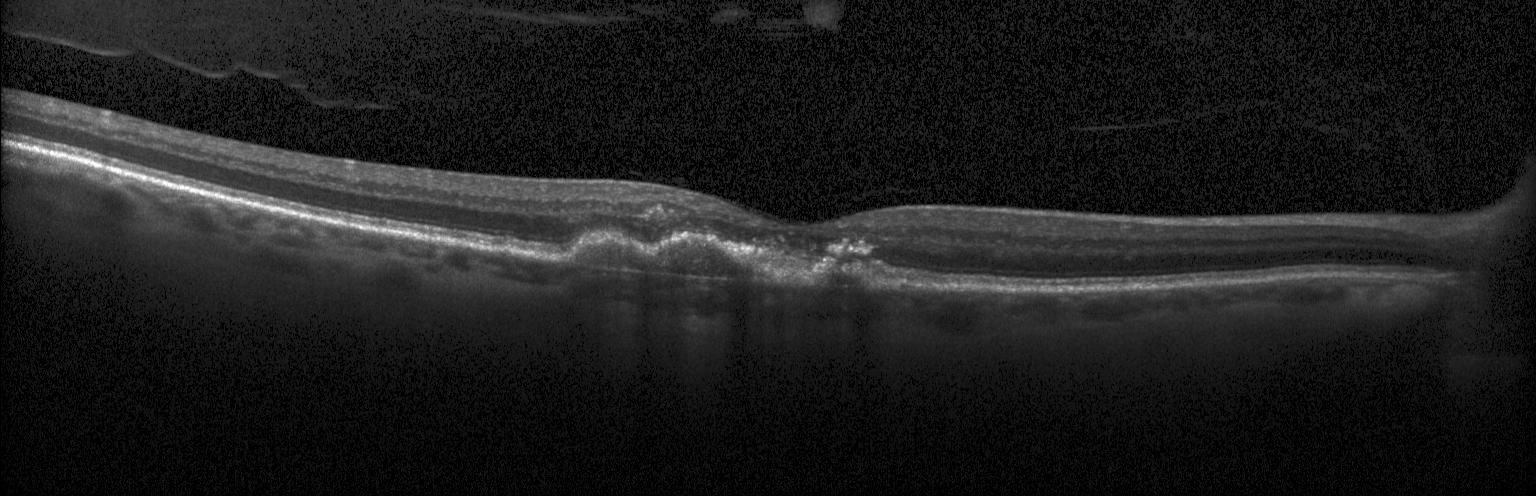 Finding: a choroidal neovascular membrane.